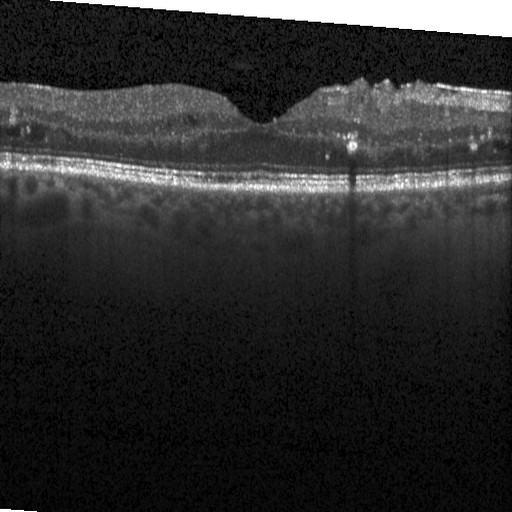

The scan shows DME.